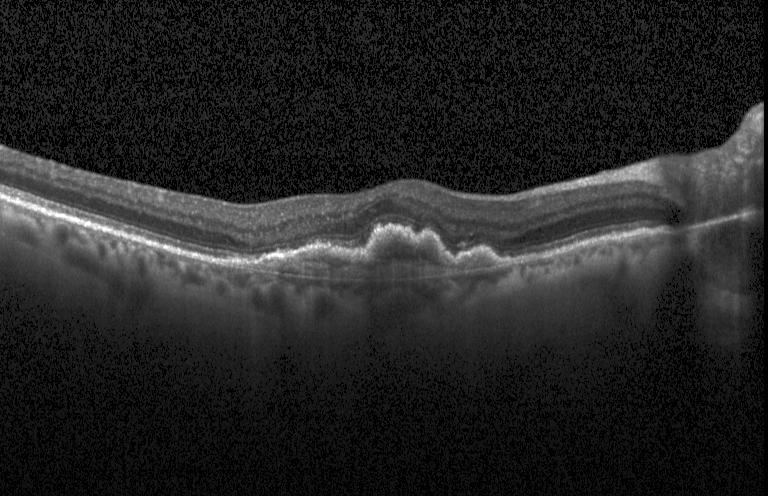

Diagnosis: choroidal neovascularization.